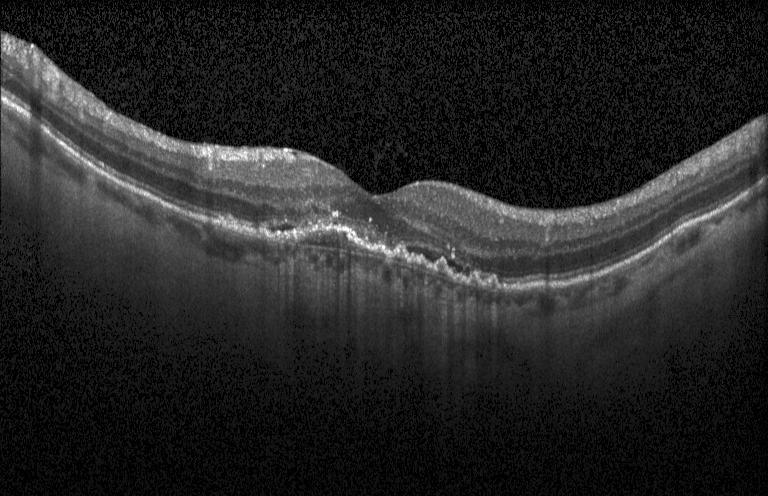 Finding: choroidal neovascularization (CNV).